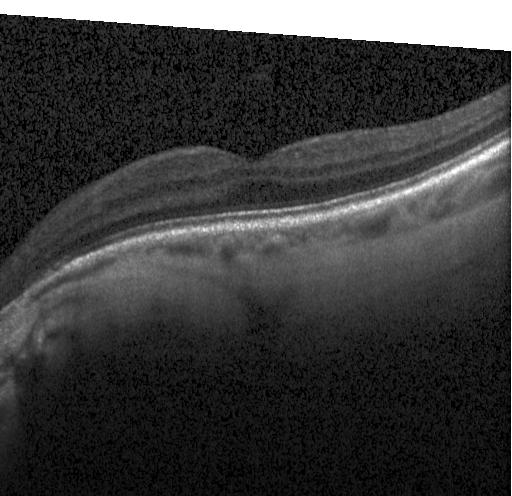

No evidence of choroidal neovascularization, diabetic macular edema, or drusen.